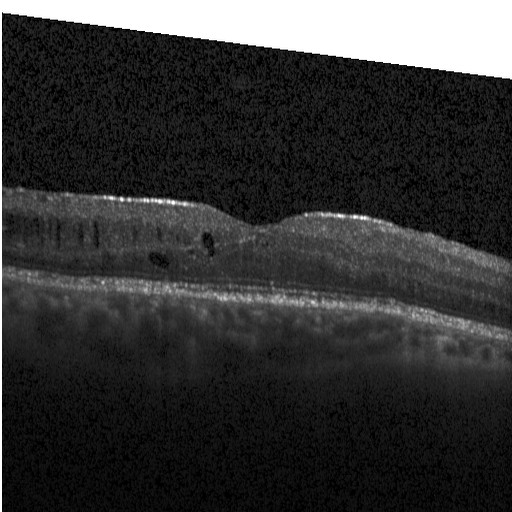
Diagnosis: DME.